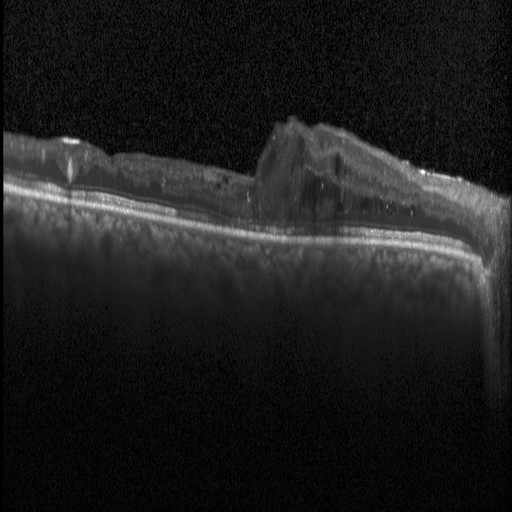
Through the macula, acquired on a Heidelberg Spectralis, spectral-domain OCT, optical coherence tomography B-scan — Diabetic macular edema (DME).